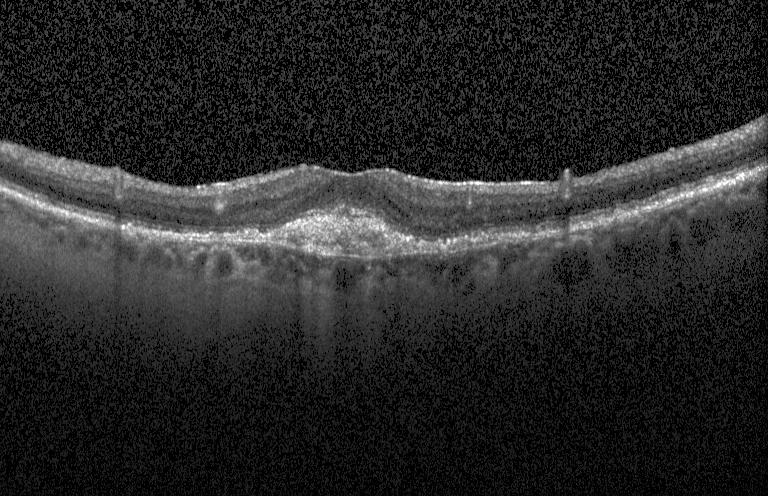

Retinal OCT B-scan
The scan shows choroidal neovascularization.